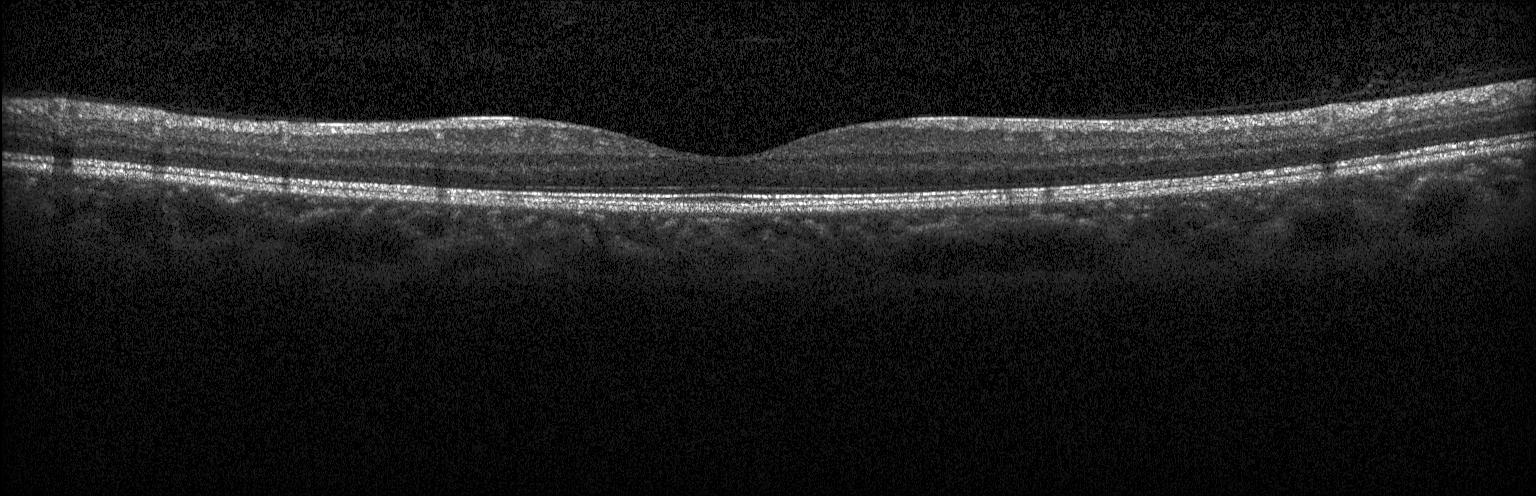 OCT line scan.
Neither choroidal neovascularization, diabetic macular edema, nor drusen.